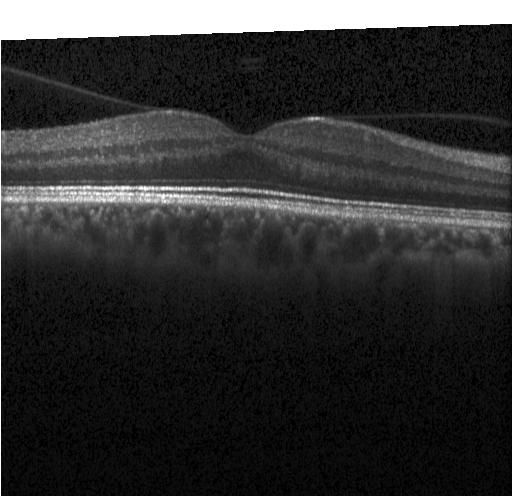
Spectral-domain optical coherence tomography · OCT line scan — No choroidal neovascularization, diabetic macular edema, or drusen.